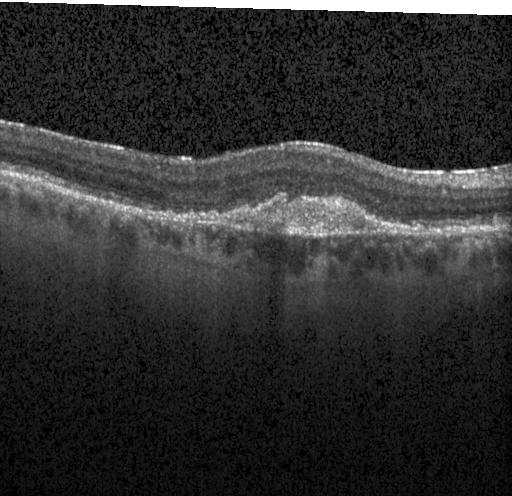
OCT B-scan
Impression: a choroidal neovascular membrane.